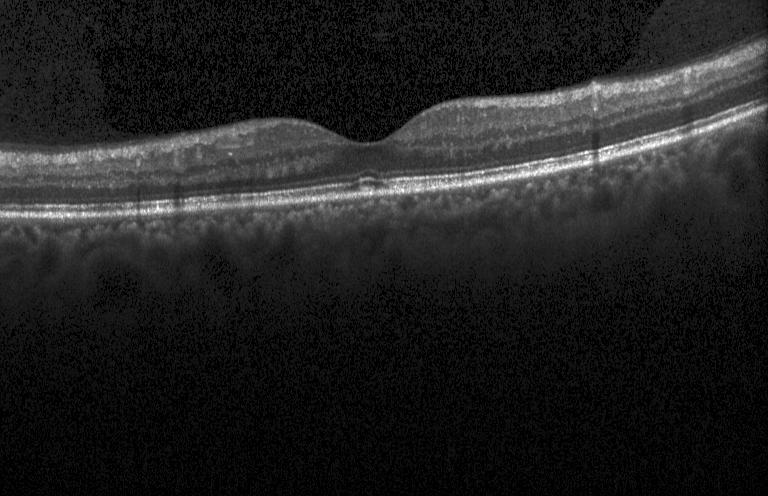

Spectral-domain OCT B-scan: neither CNV, DME, nor drusen.